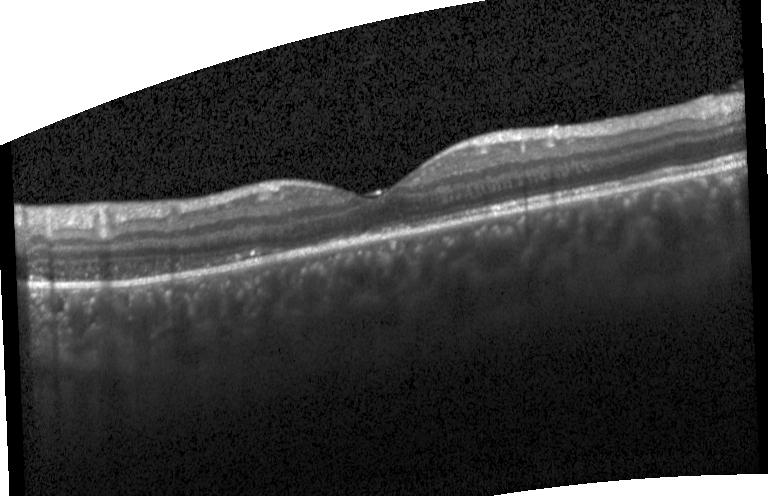 Heidelberg Spectralis · through the macula · OCT B-scan · spectral-domain optical coherence tomography
Diagnosis: neither choroidal neovascularization, diabetic macular edema, nor drusen.